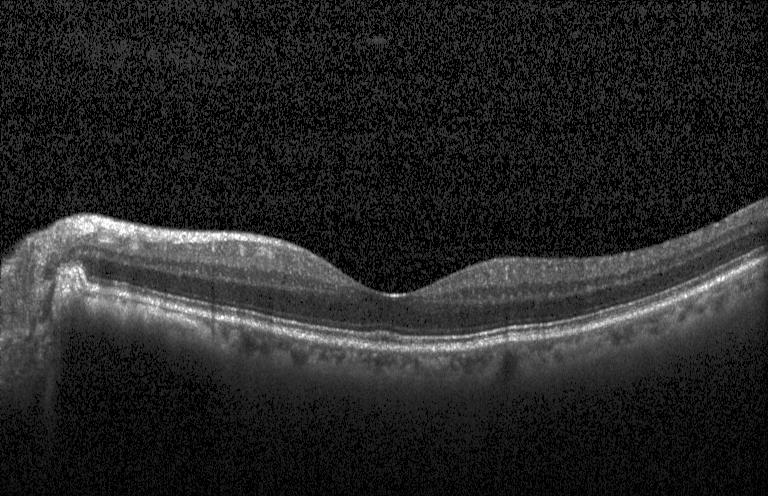

Retinal OCT B-scan · SD-OCT · horizontal scan through the fovea · Heidelberg Spectralis OCT system — The scan shows no CNV, DME, or drusen.